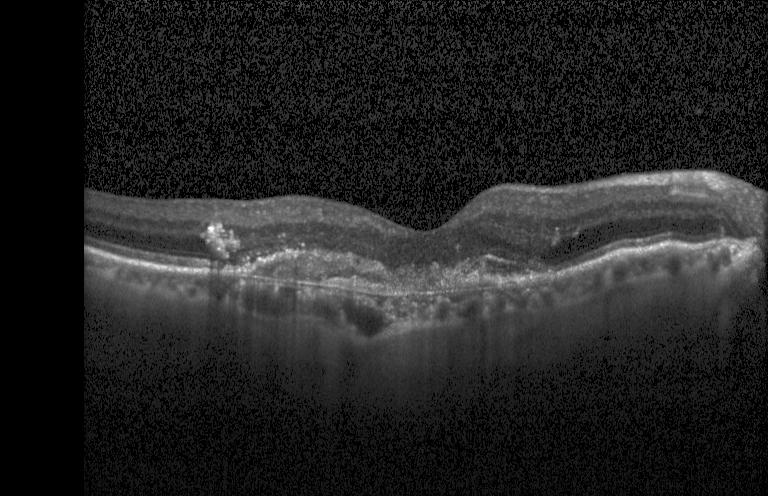
Acquired on a Heidelberg Spectralis, OCT B-scan, spectral-domain optical coherence tomography, macular scan. Impression: choroidal neovascularization.